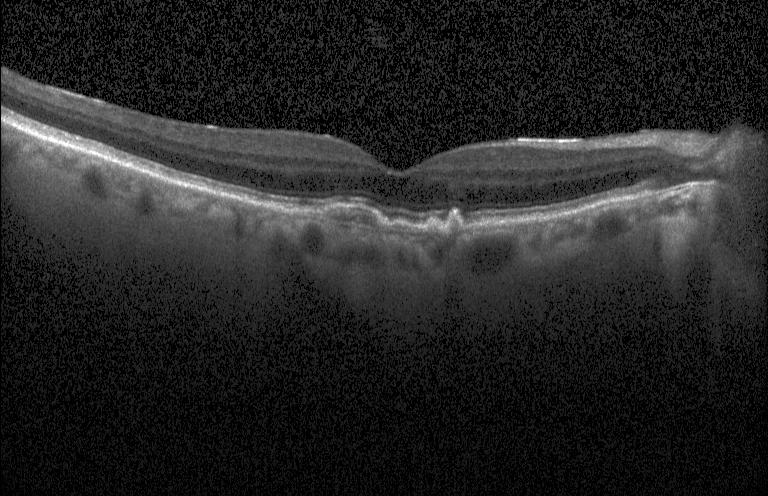

Retinal OCT B-scan — Diagnosis: choroidal neovascularization.